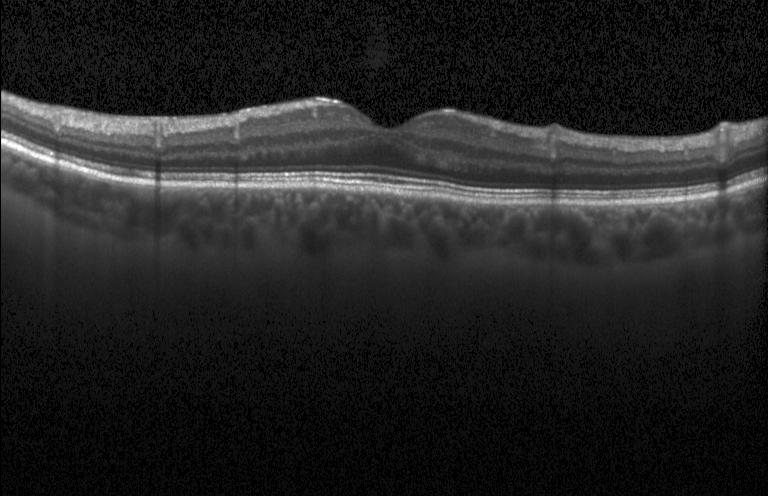

Through the macula. Spectral-domain optical coherence tomography. Retinal OCT cross-section.
Finding: no choroidal neovascularization, no diabetic macular edema, and no drusen.